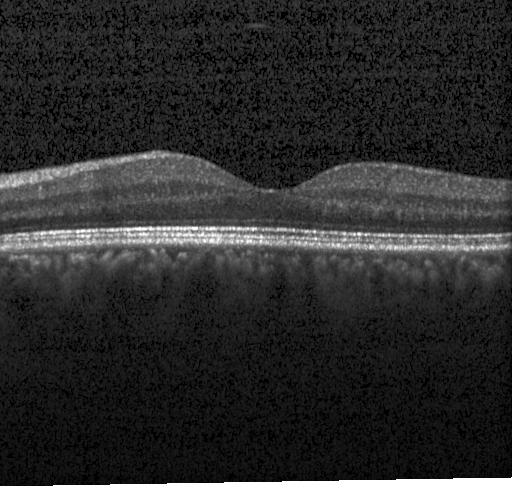
OCT line scan. Dx: no evidence of choroidal neovascularization, diabetic macular edema, or drusen.